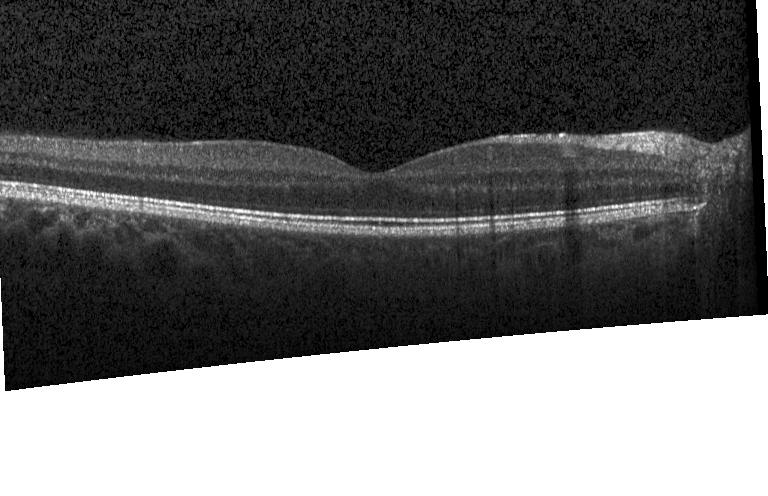 Heidelberg Spectralis OCT system, fovea-centered, OCT B-scan
Diagnosis: no CNV, no DME, and no drusen.